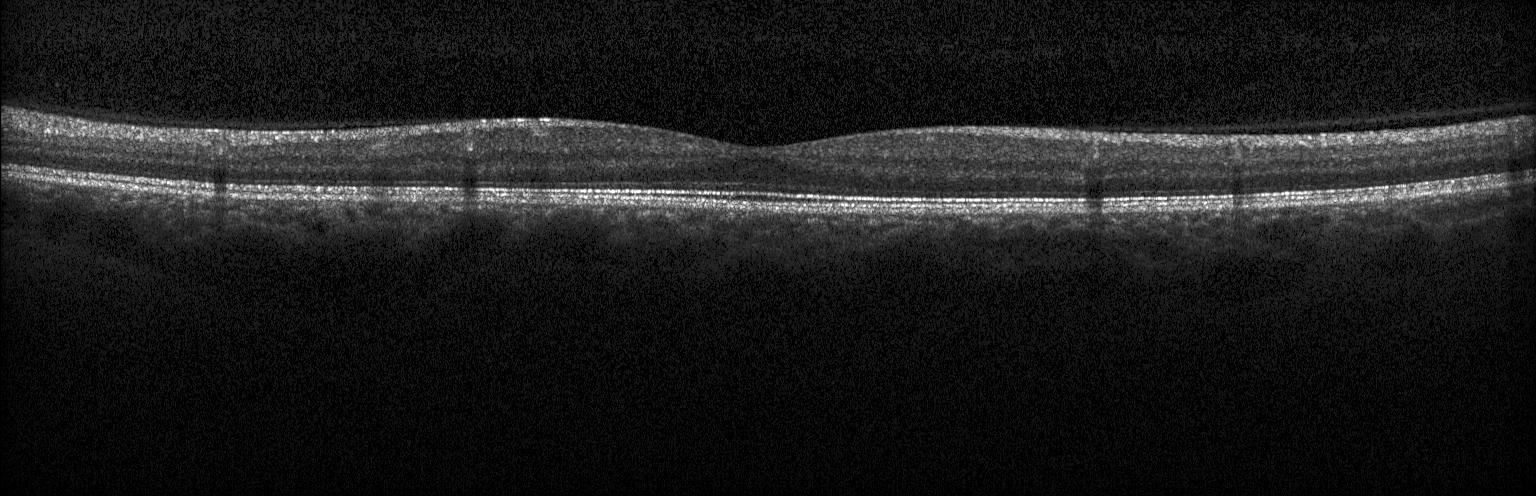

Macular OCT demonstrating no evidence of choroidal neovascularization, diabetic macular edema, or drusen.